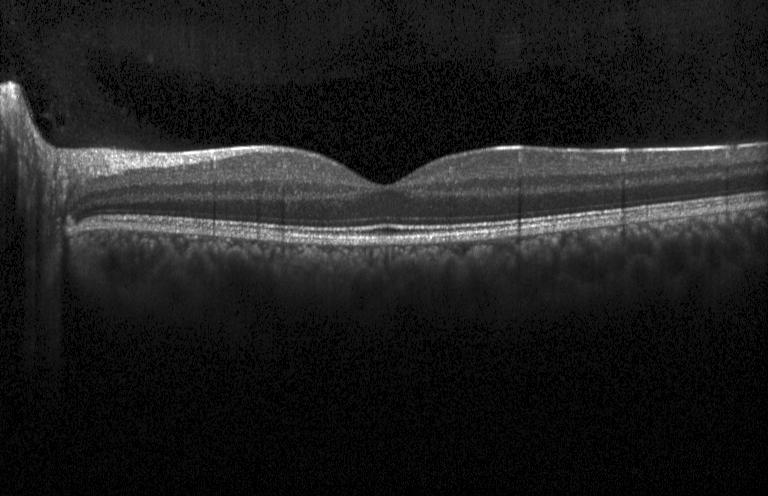
Spectral-domain optical coherence tomography · optical coherence tomography scan. OCT finding: no evidence of CNV, DME, or drusen.